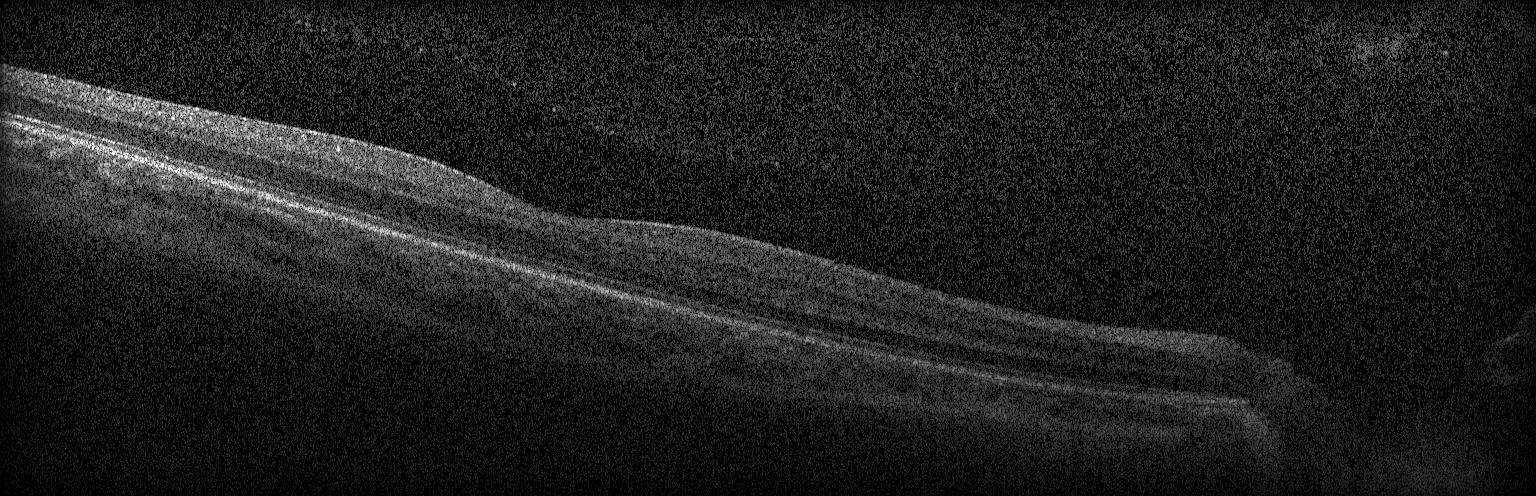

Spectral-domain OCT B-scan: no choroidal neovascularization, no diabetic macular edema, and no drusen.